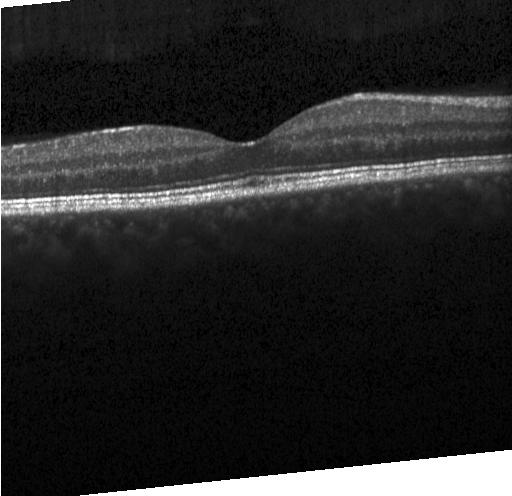 OCT line scan; Heidelberg Spectralis OCT system; spectral-domain optical coherence tomography.
Finding: no CNV, DME, or drusen.